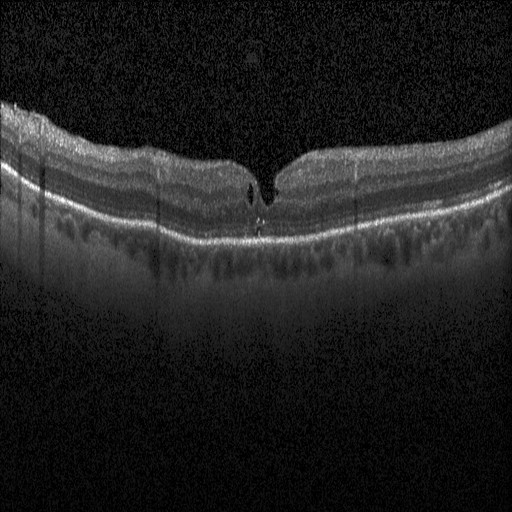

Through the macula; OCT B-scan; instrument: Heidelberg Spectralis; spectral-domain optical coherence tomography. Finding: DME.